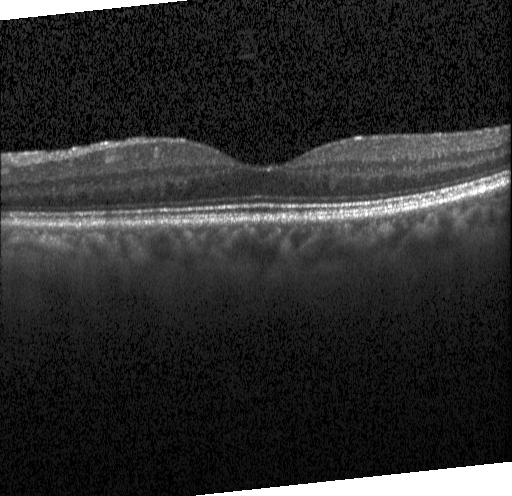
Fovea-centered. OCT B-scan. The scan shows no CNV, DME, or drusen.